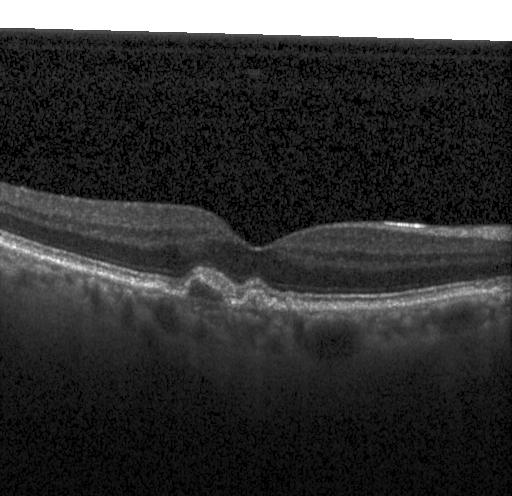
Spectral-domain optical coherence tomography. OCT B-scan.
Macular OCT: CNV.